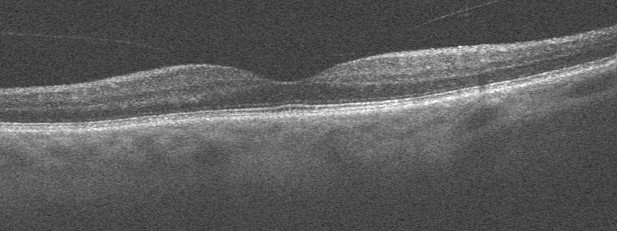

OCT B-scan showing absence of AMD, DME, ERM, RAO, RVO, and vitreomacular interface disease.